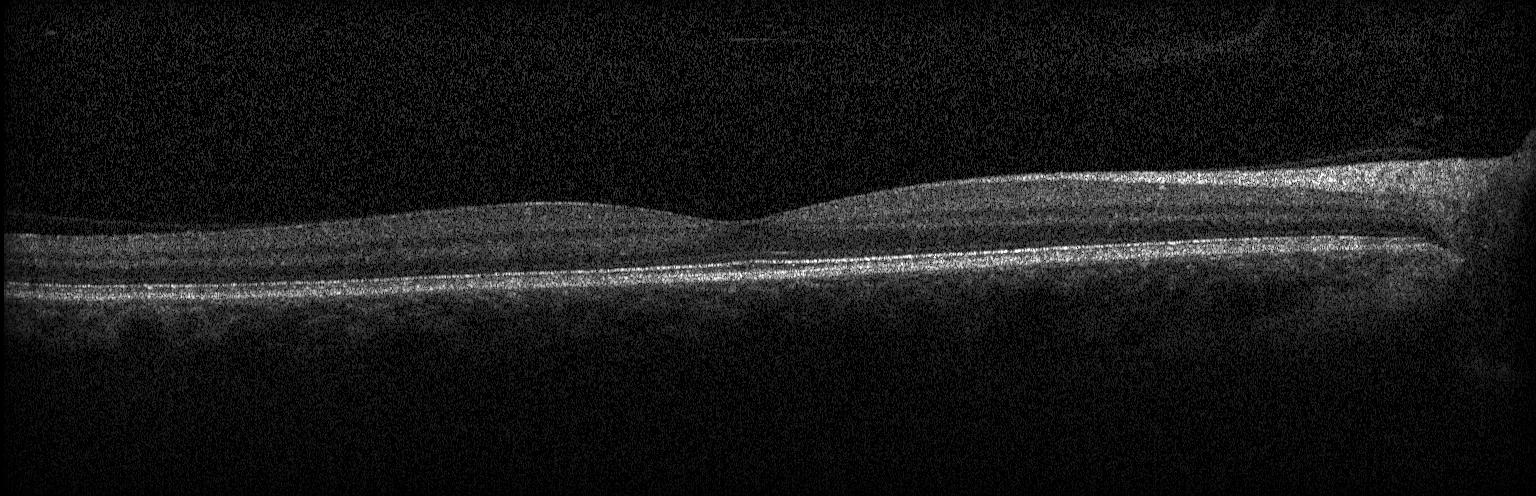 Spectral-domain OCT B-scan: neither CNV, DME, nor drusen.